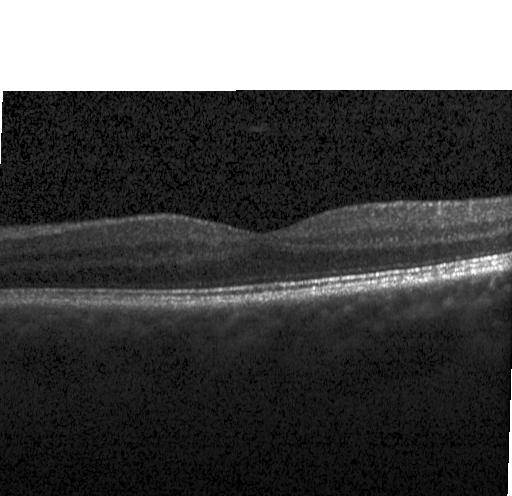 Retinal OCT cross-section. Through the macula. Heidelberg Spectralis OCT system. Finding: neither choroidal neovascularization, diabetic macular edema, nor drusen.